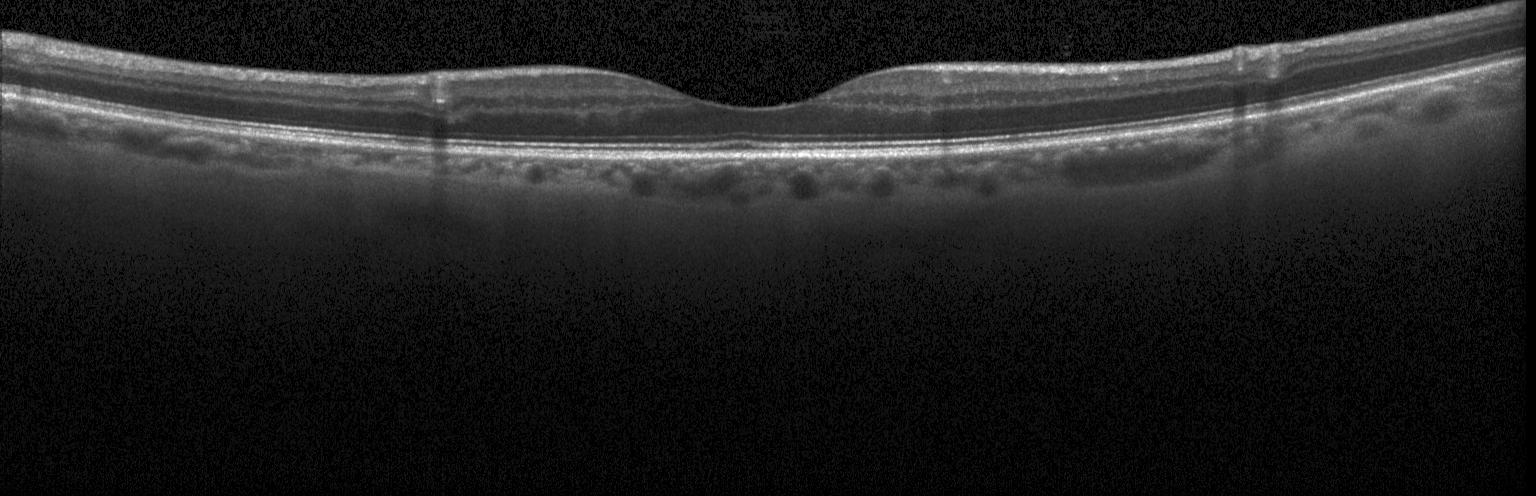
Assessment: no evidence of choroidal neovascularization, diabetic macular edema, or drusen.